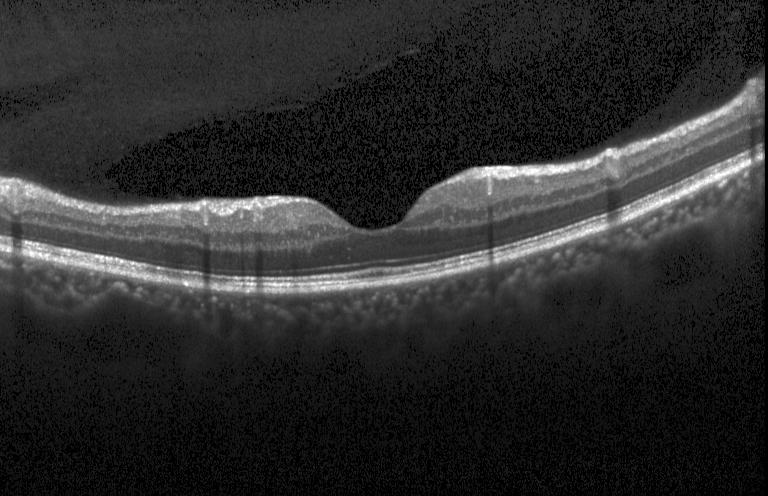 OCT line scan · centered on the fovea · SD-OCT · Heidelberg Spectralis OCT system.
Diagnosis: neither CNV, DME, nor drusen.